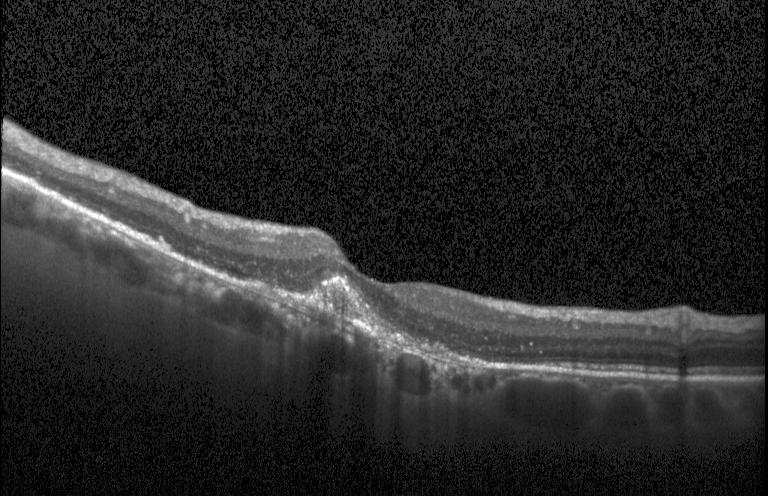
Macular OCT: a choroidal neovascular membrane.